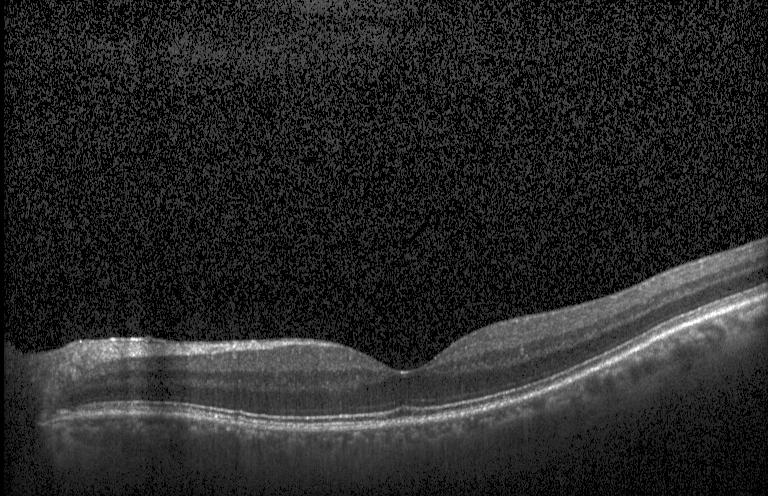

Impression: no evidence of choroidal neovascularization, diabetic macular edema, or drusen.